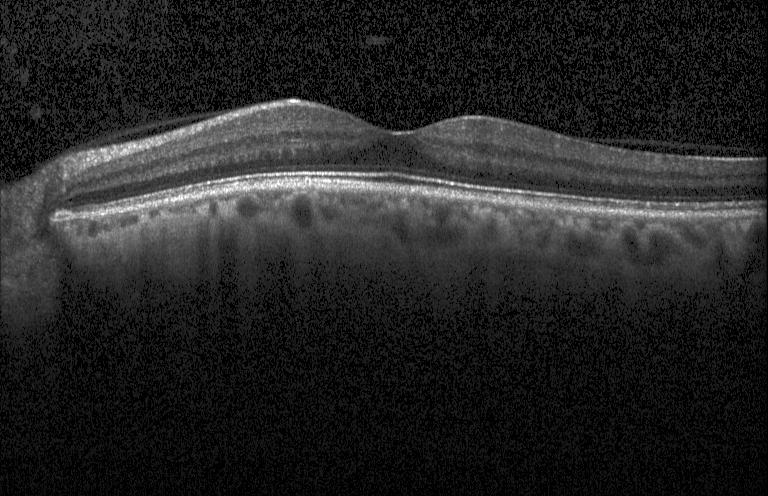
OCT B-scan showing no choroidal neovascularization, no diabetic macular edema, and no drusen.